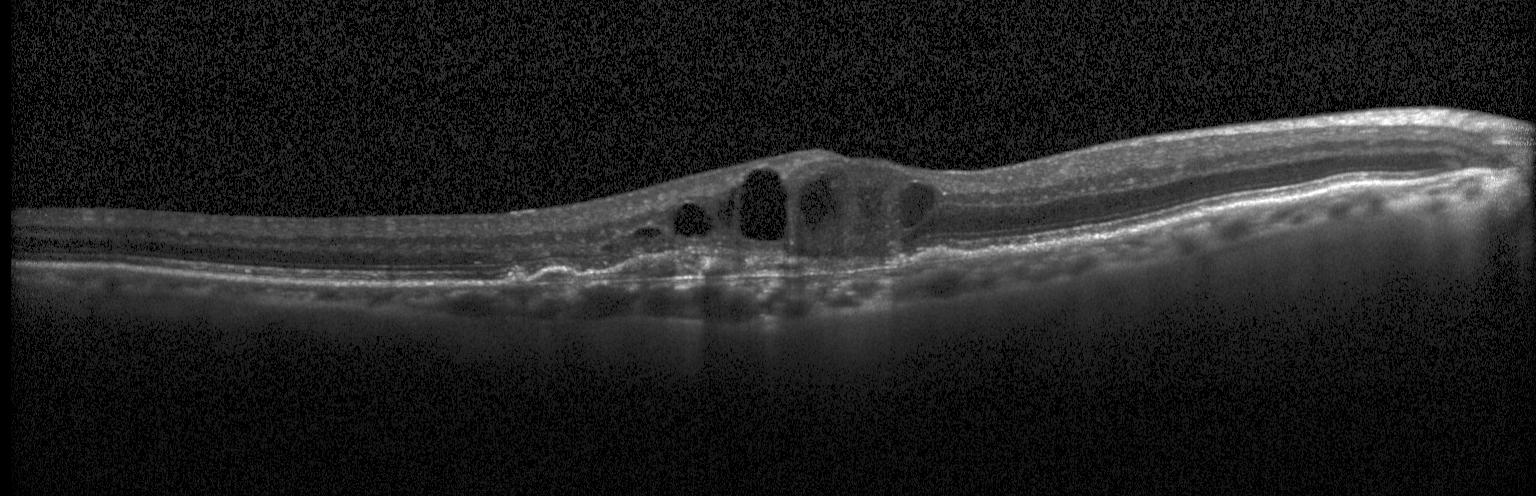

Retinal OCT cross-section, Heidelberg Spectralis.
Impression: CNV.